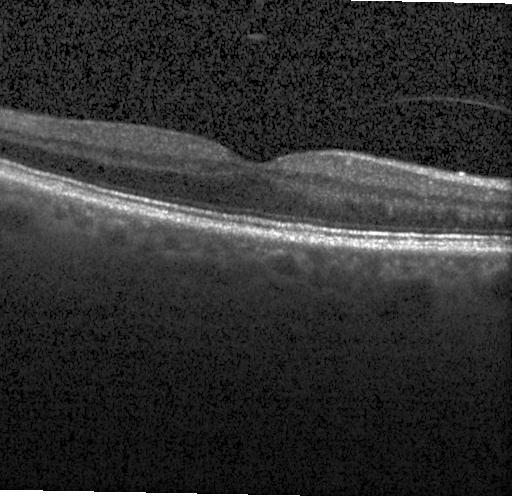
OCT finding: no choroidal neovascularization, diabetic macular edema, or drusen.